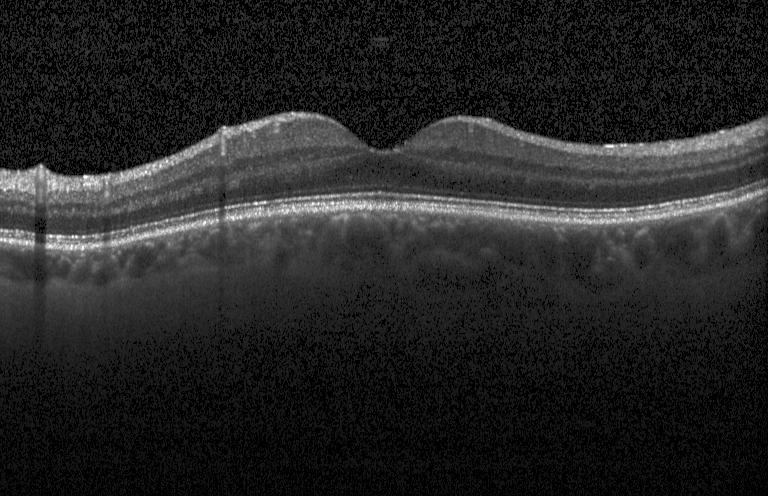

Spectral-domain OCT · retinal OCT cross-section · through the macula.
Macular OCT: neither choroidal neovascularization, diabetic macular edema, nor drusen.